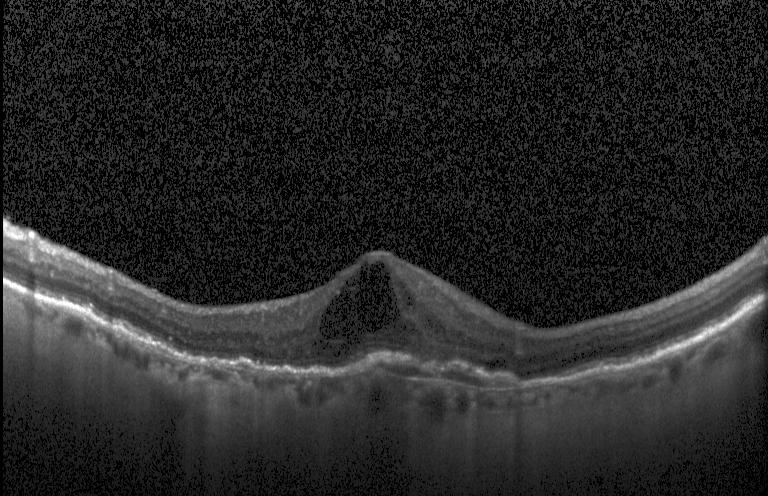 Optical coherence tomography B-scan; SD-OCT; Heidelberg Spectralis; horizontal scan through the fovea — Impression: choroidal neovascularization.